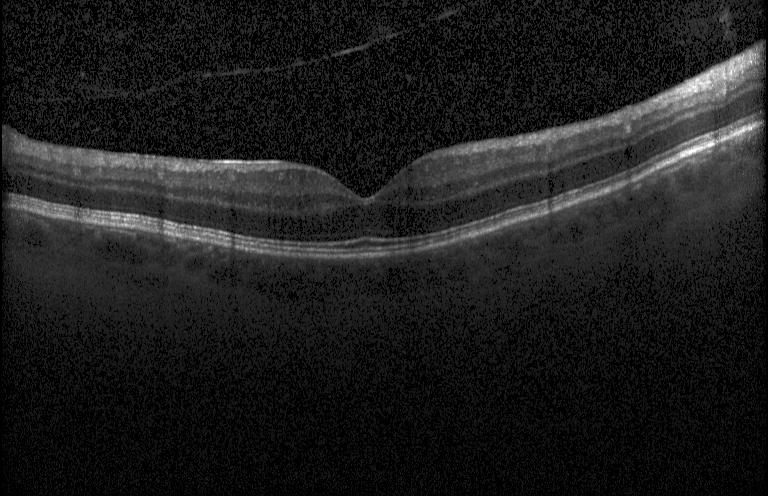 This B-scan demonstrates neither CNV, DME, nor drusen.